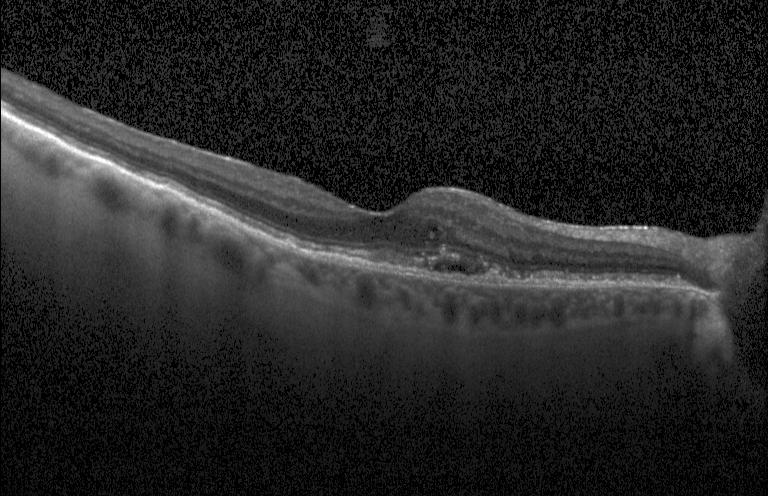
Acquired on a Heidelberg Spectralis, OCT B-scan, fovea-centered, spectral-domain OCT
OCT finding: a choroidal neovascular membrane.